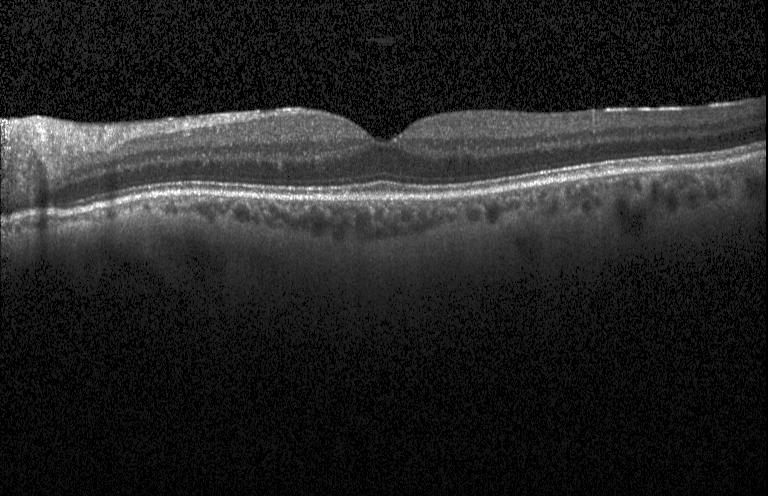 Macular scan. Retinal OCT cross-section — Diagnosis: no choroidal neovascularization, diabetic macular edema, or drusen.